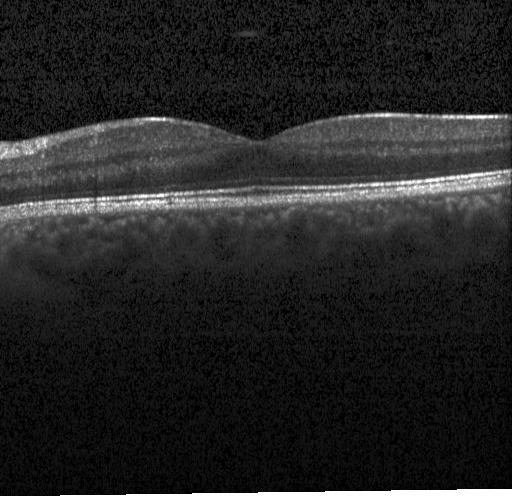 Dx: no CNV, DME, or drusen.